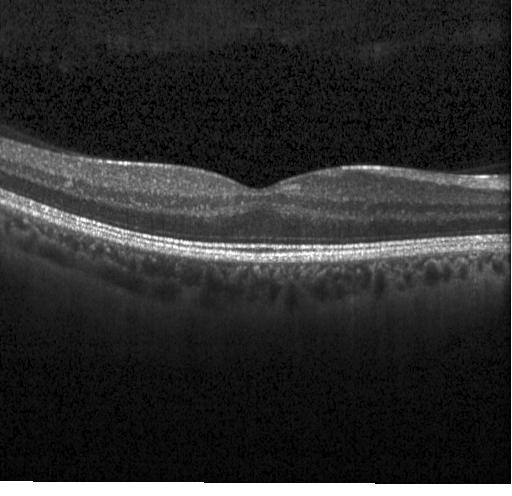 Retinal OCT B-scan
Impression: no evidence of CNV, DME, or drusen.